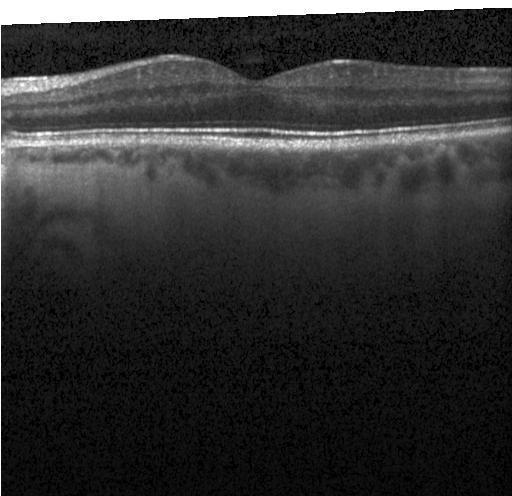

Retinal OCT B-scan.
Diagnosis: no evidence of choroidal neovascularization, diabetic macular edema, or drusen.